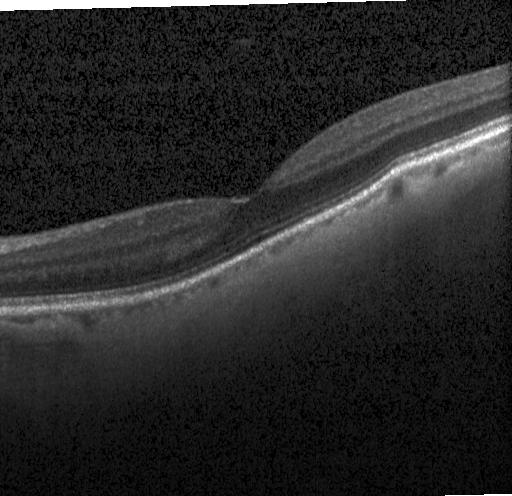 Finding: no CNV, no DME, and no drusen.